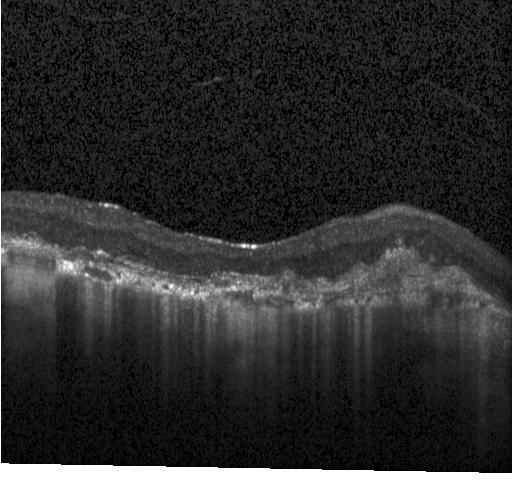

OCT line scan; spectral-domain OCT.
Macular OCT: choroidal neovascularization.